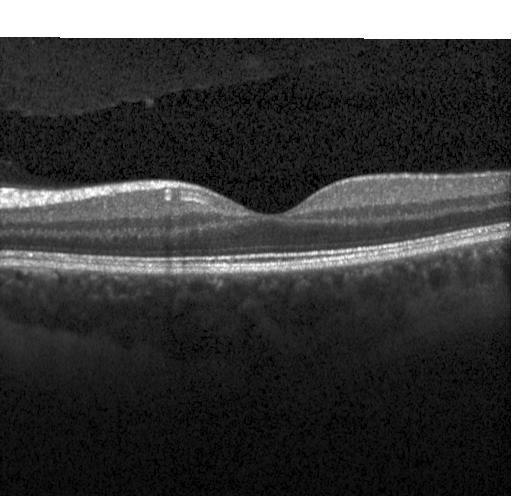

OCT finding: no evidence of CNV, DME, or drusen.